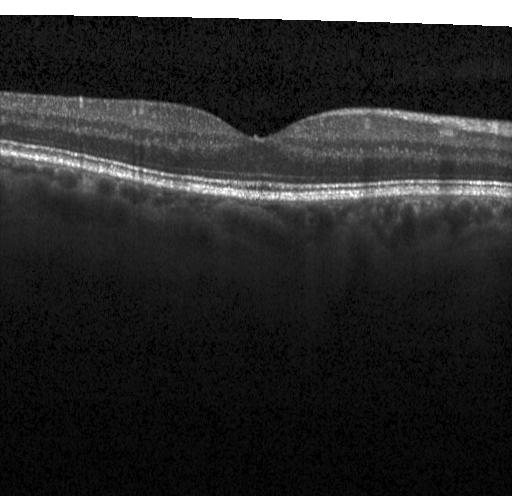

OCT line scan. Spectral-domain optical coherence tomography. Fovea-centered.
This B-scan demonstrates no CNV, DME, or drusen.